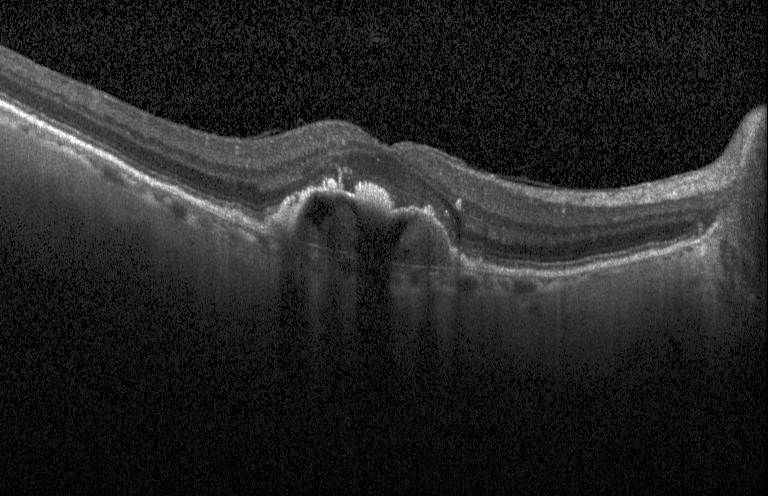 Finding: choroidal neovascularization (CNV).